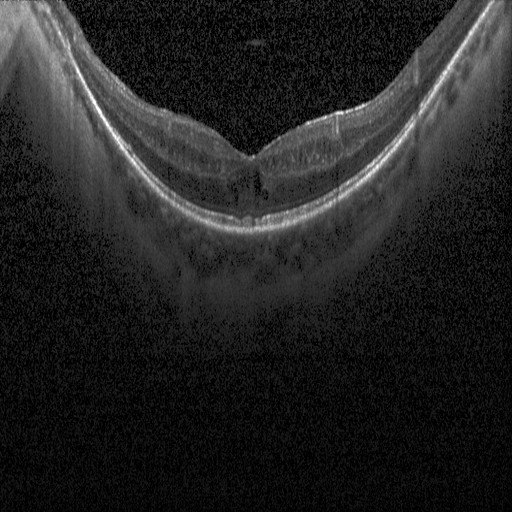 This B-scan demonstrates DME.